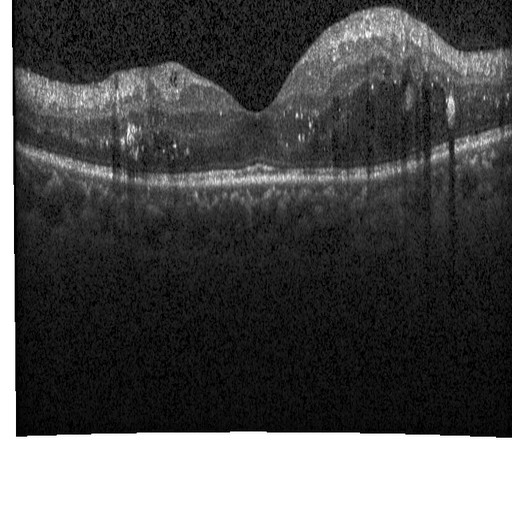
Retinal OCT cross-section; acquired on a Heidelberg Spectralis; through the macula.
Finding: diabetic macular edema (DME).